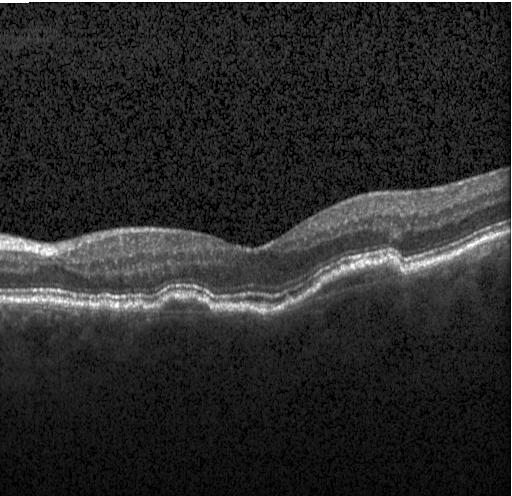

Acquired on a Heidelberg Spectralis · SD-OCT · through the macula · OCT line scan — Diagnosis: a choroidal neovascular membrane.